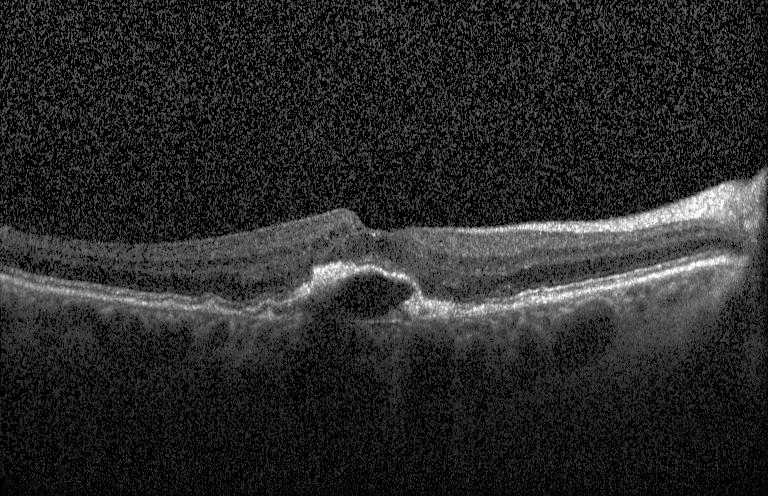

Spectral-domain optical coherence tomography, Heidelberg Spectralis, retinal OCT cross-section, macular scan.
The scan shows a choroidal neovascular membrane.